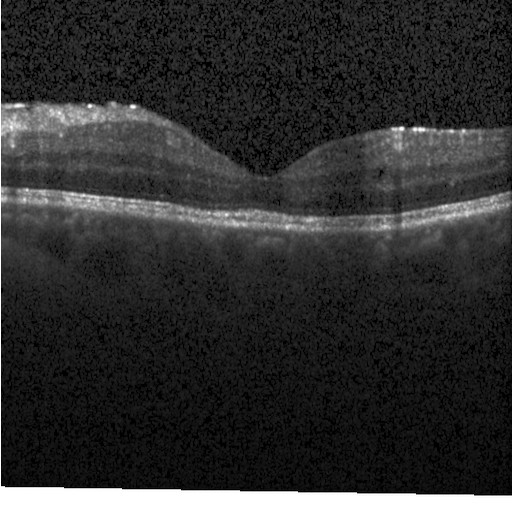 Retinal OCT B-scan. Diagnosis: DME.